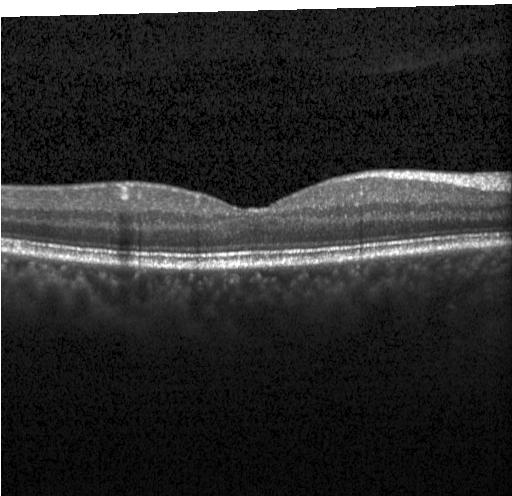 OCT B-scan showing neither choroidal neovascularization, diabetic macular edema, nor drusen.